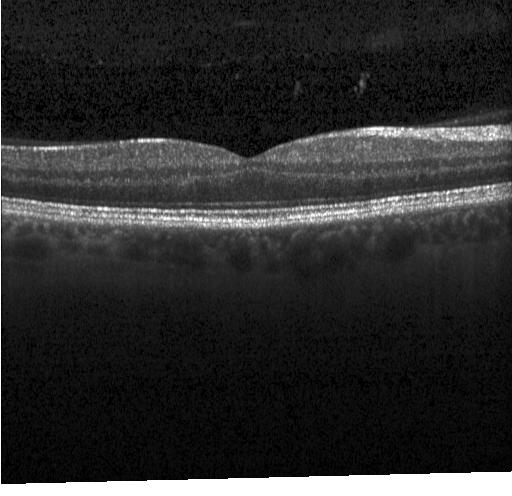

OCT B-scan — This B-scan demonstrates neither CNV, DME, nor drusen.